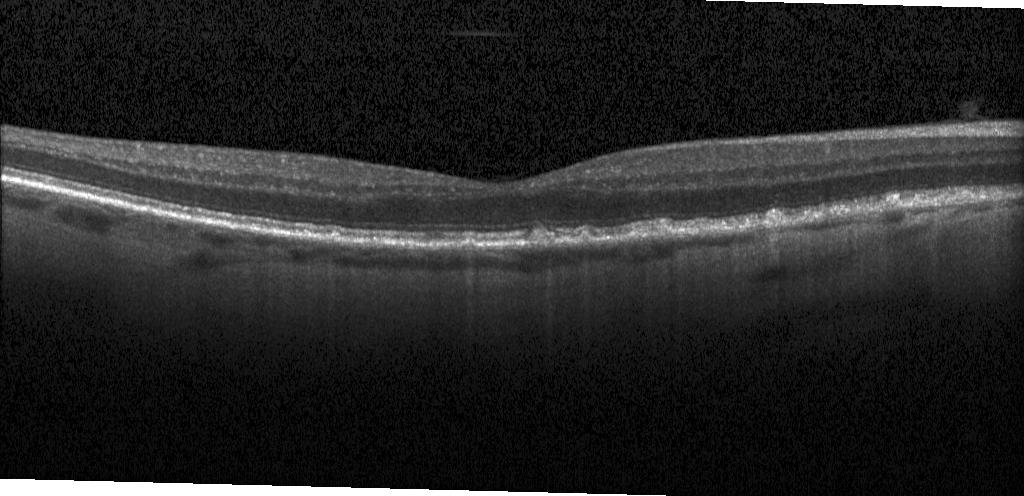

Impression: drusen.